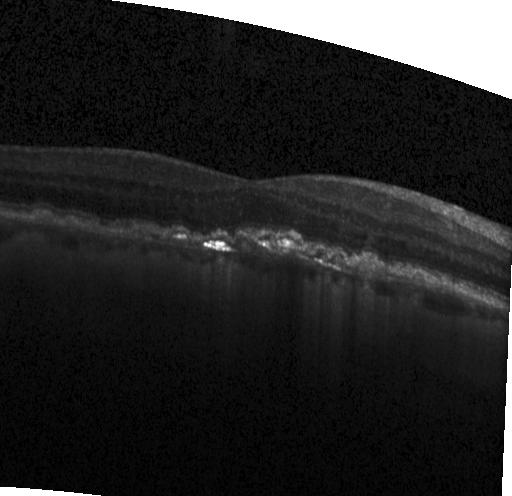 Fovea-centered, optical coherence tomography scan. Dx: a choroidal neovascular membrane.